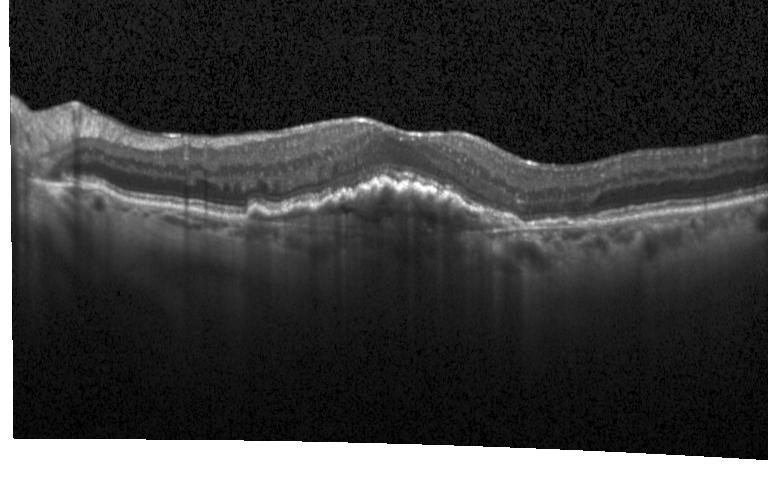 OCT line scan
Macular OCT: choroidal neovascularization.